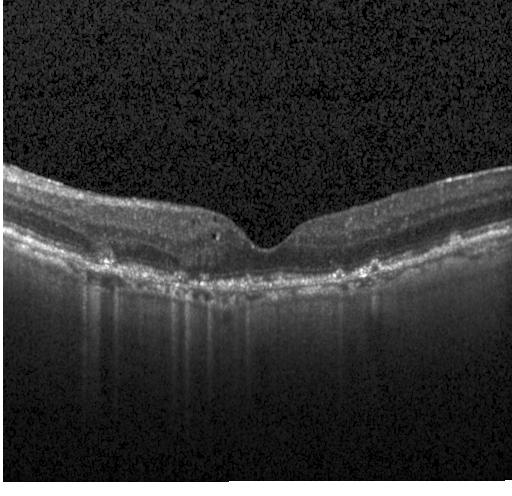

OCT B-scan, through the macula, instrument: Heidelberg Spectralis, spectral-domain OCT
Dx: a choroidal neovascular membrane.